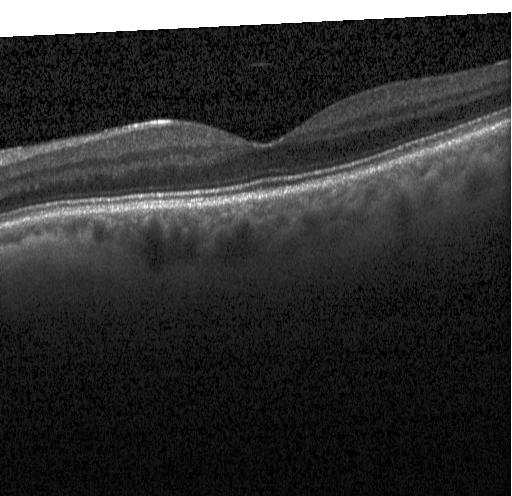 Optical coherence tomography B-scan.
Impression: no choroidal neovascularization, diabetic macular edema, or drusen.